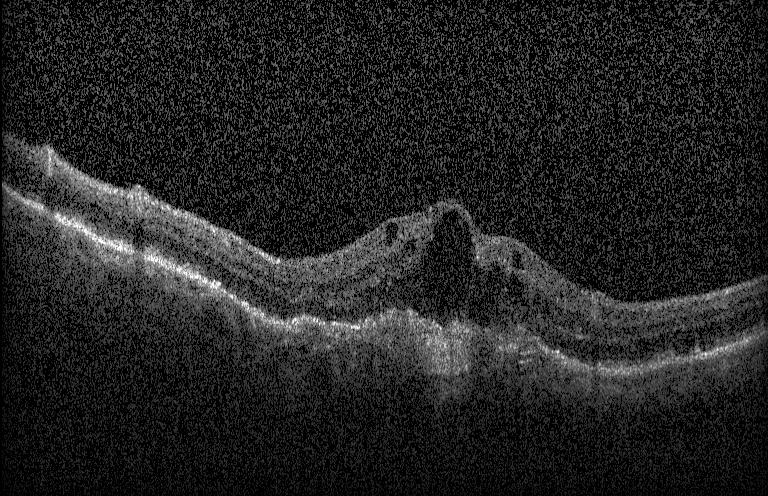 SD-OCT; Heidelberg Spectralis; retinal OCT cross-section.
Finding: a choroidal neovascular membrane.